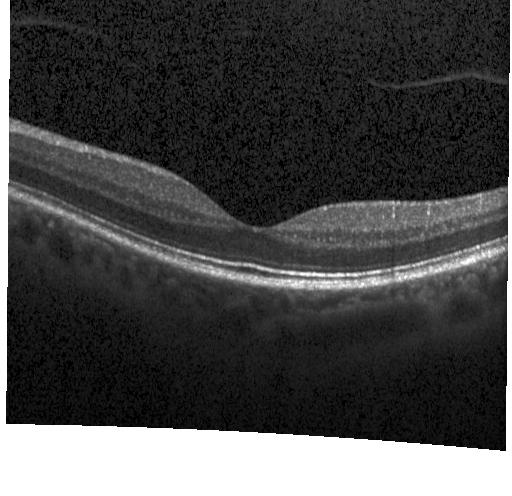

OCT B-scan. Finding: no CNV, DME, or drusen.